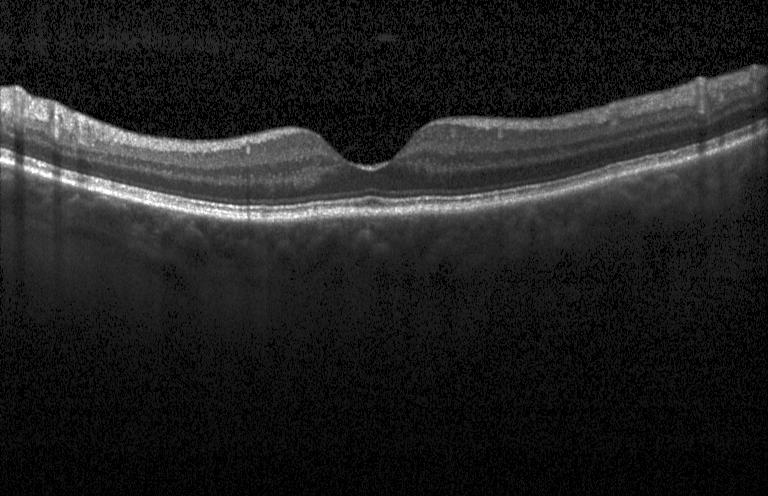 Impression: no CNV, DME, or drusen.